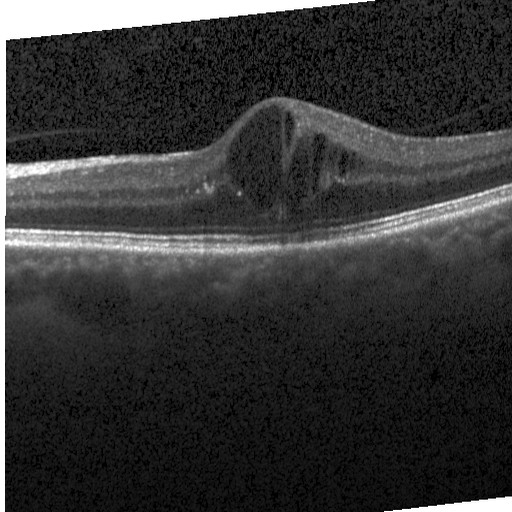
Retinal OCT cross-section · centered on the fovea · Heidelberg Spectralis · spectral-domain optical coherence tomography. Finding: diabetic macular edema.